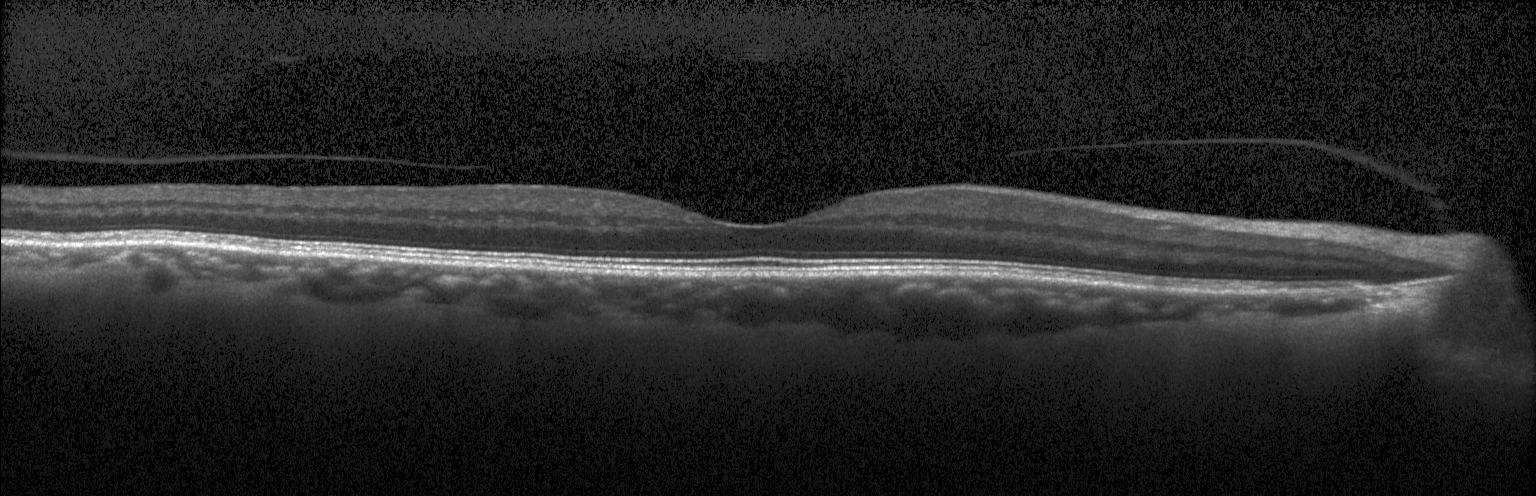
Horizontal scan through the fovea. Retinal OCT B-scan — Dx: no choroidal neovascularization, no diabetic macular edema, and no drusen.